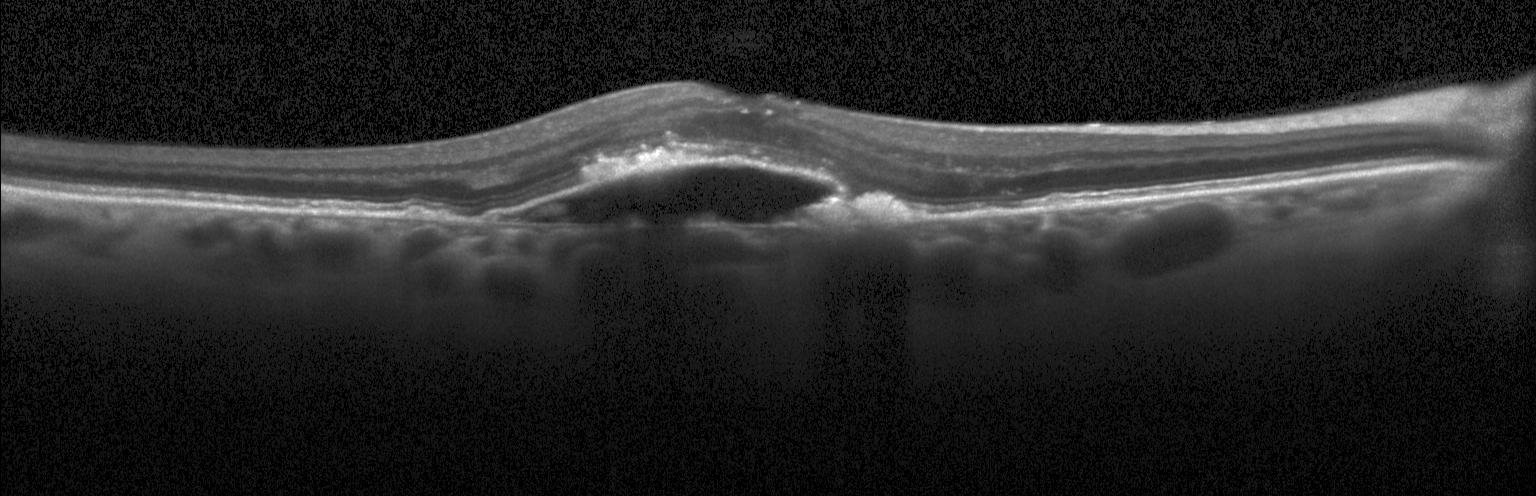 Optical coherence tomography scan, SD-OCT, Heidelberg Spectralis OCT system — Finding: CNV.